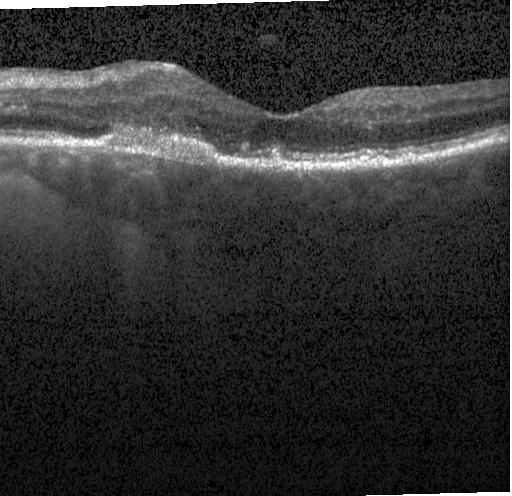

Retinal OCT cross-section showing a choroidal neovascular membrane.